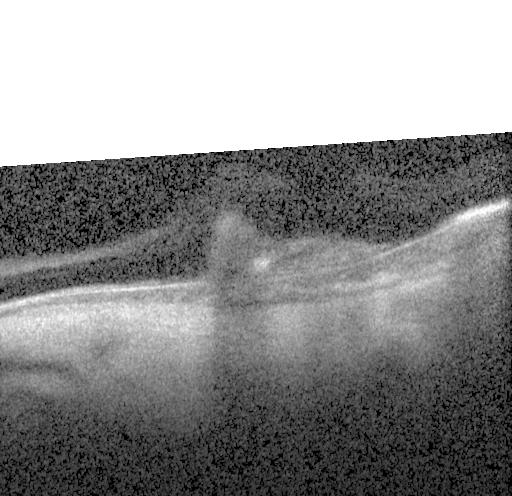

OCT scan showing choroidal neovascularization (CNV).